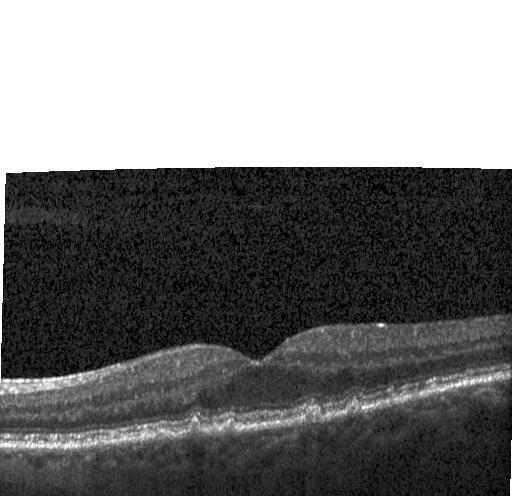 Finding: multiple drusen.